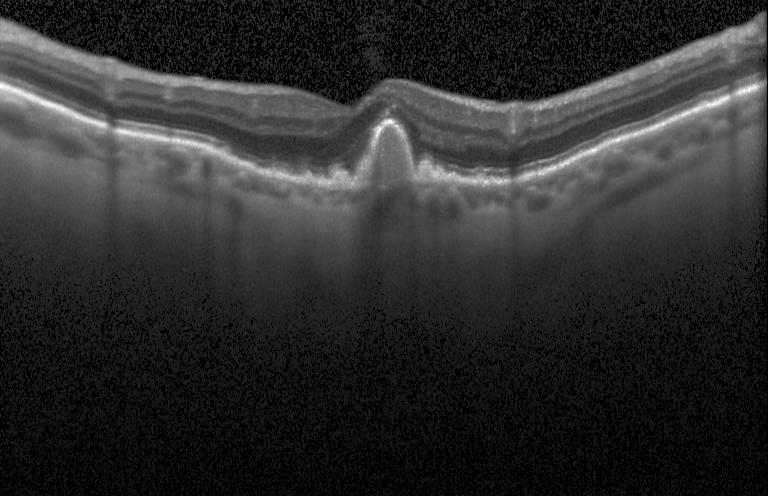

Instrument: Heidelberg Spectralis · horizontal scan through the fovea · retinal OCT cross-section · SD-OCT — Diagnosis: sub-RPE drusenoid deposits.